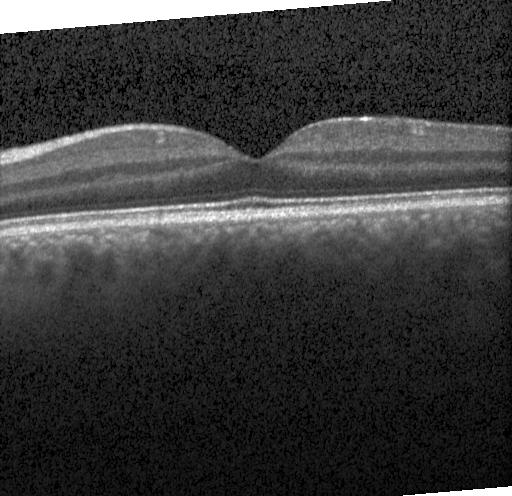
Assessment: neither CNV, DME, nor drusen.